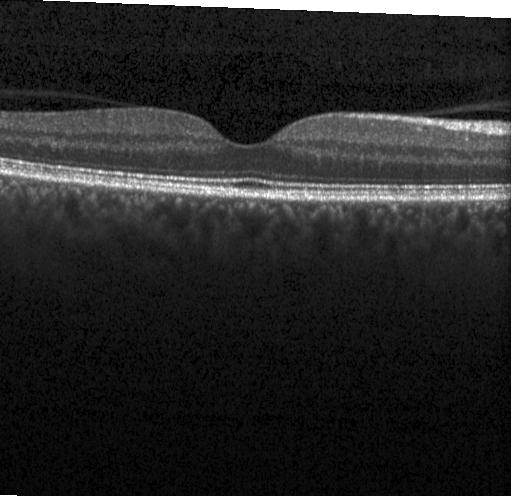
Diagnosis: no evidence of CNV, DME, or drusen.